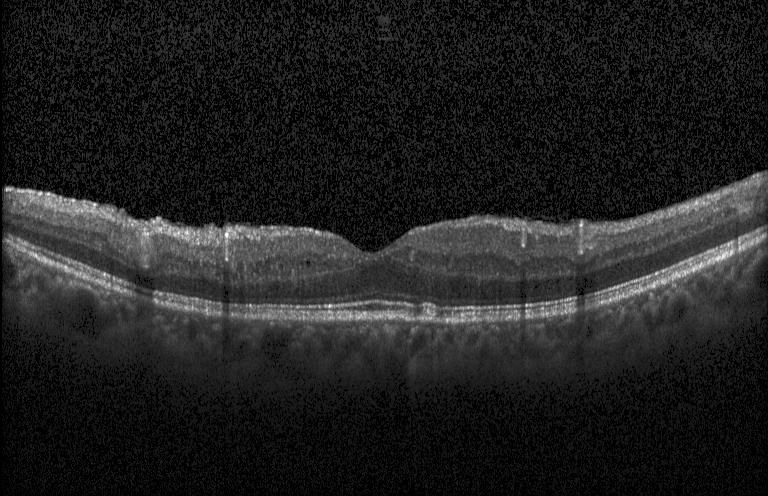

OCT line scan; Heidelberg Spectralis OCT system; SD-OCT
Finding: DME.